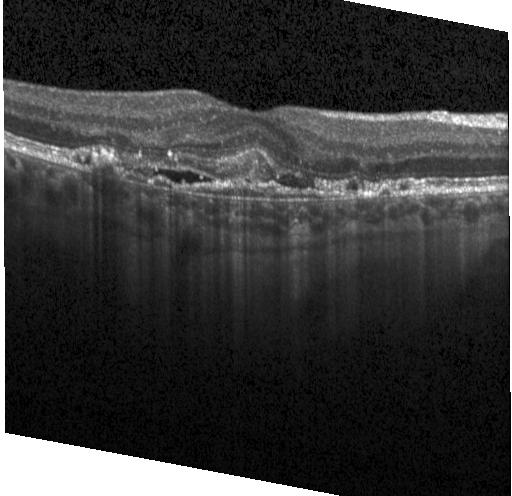
Finding: a choroidal neovascular membrane.